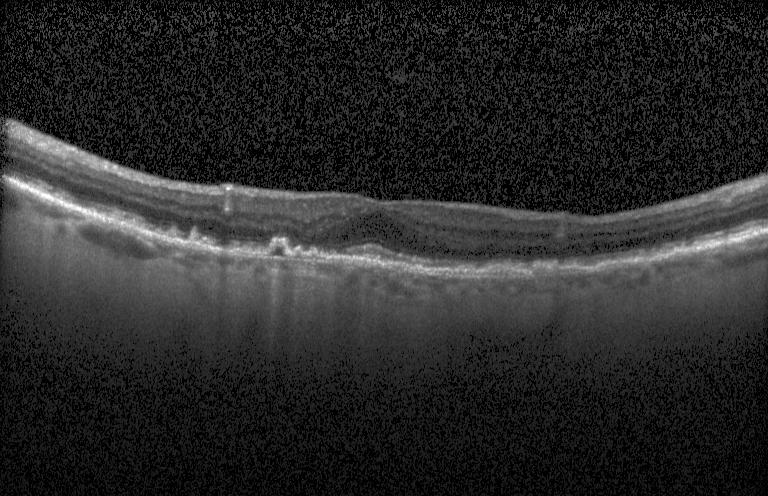
The scan shows drusen.